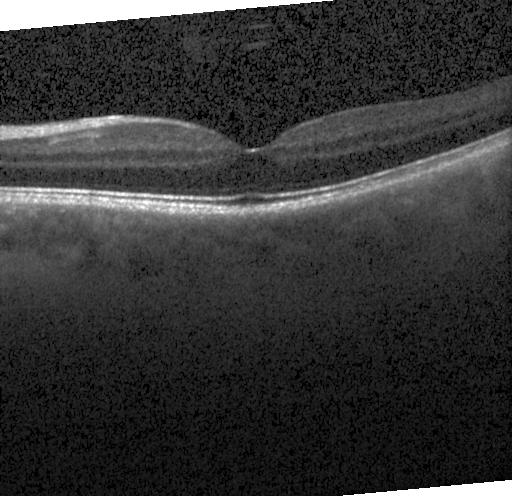
Through the macula. Retinal OCT cross-section.
Finding: no CNV, no DME, and no drusen.